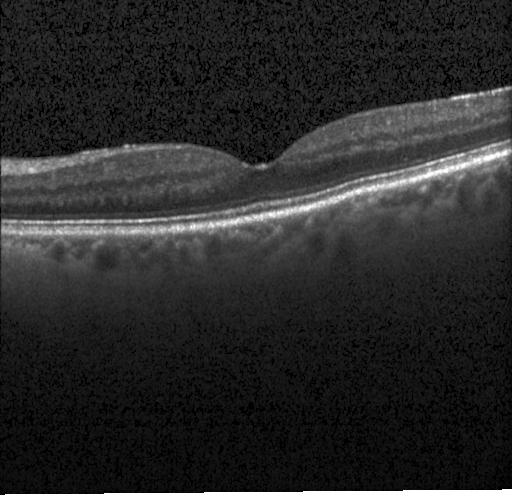

This B-scan demonstrates no evidence of choroidal neovascularization, diabetic macular edema, or drusen.